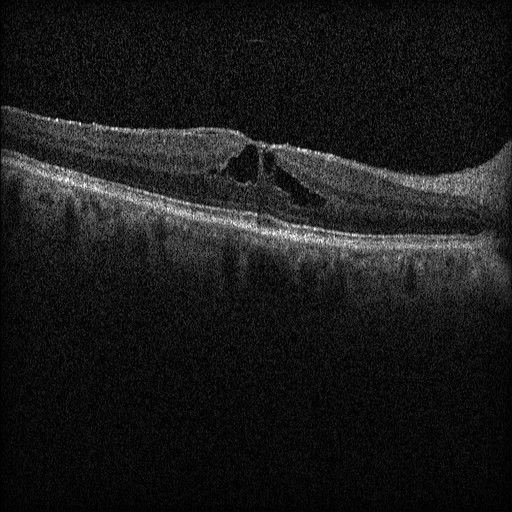 Retinal OCT cross-section showing DME.